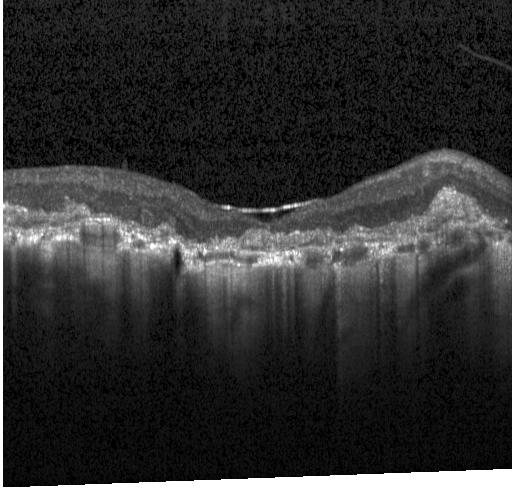

Optical coherence tomography B-scan, SD-OCT, Heidelberg Spectralis. Assessment: choroidal neovascularization (CNV).